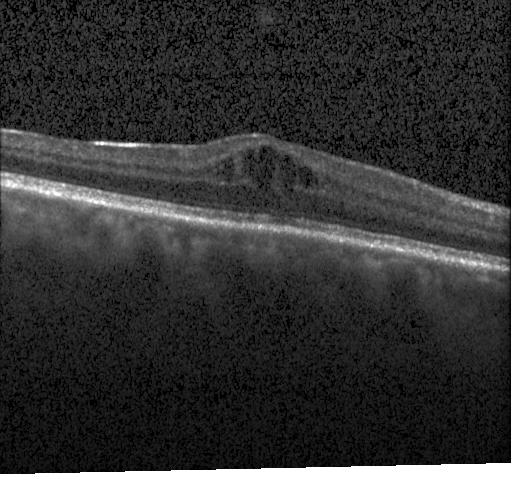

Centered on the fovea. Retinal OCT B-scan
Macular OCT: DME.